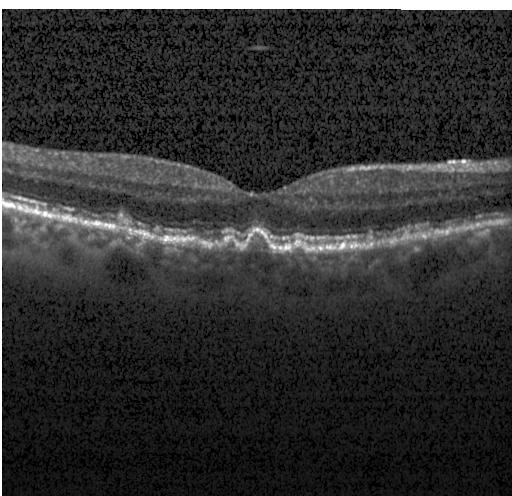

OCT line scan. Assessment: multiple drusen.